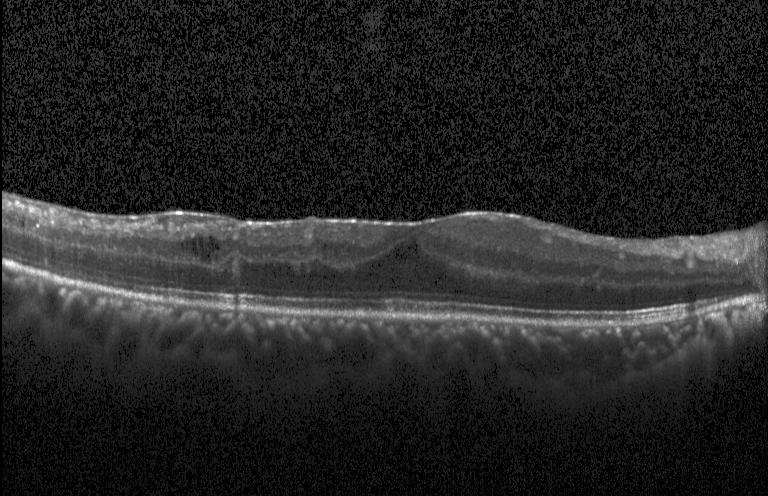
SD-OCT, through the macula, instrument: Heidelberg Spectralis, optical coherence tomography B-scan.
Assessment: diabetic macular edema (DME).